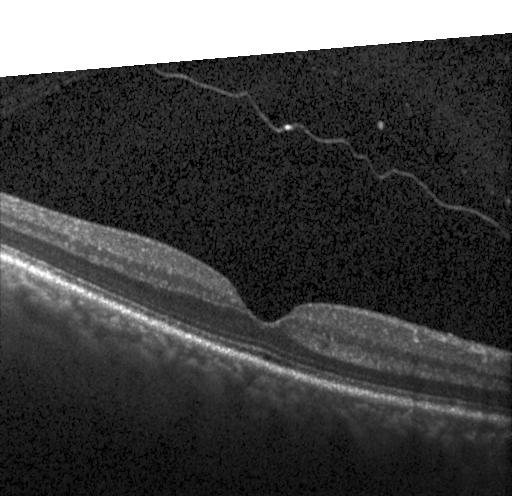

Optical coherence tomography scan; spectral-domain OCT
Finding: no choroidal neovascularization, no diabetic macular edema, and no drusen.